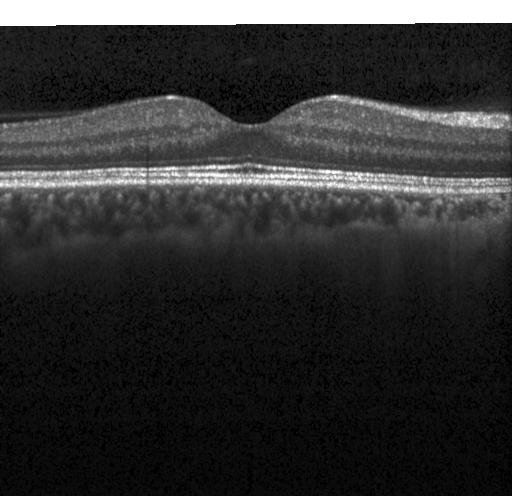
Spectral-domain OCT B-scan: no choroidal neovascularization, diabetic macular edema, or drusen.